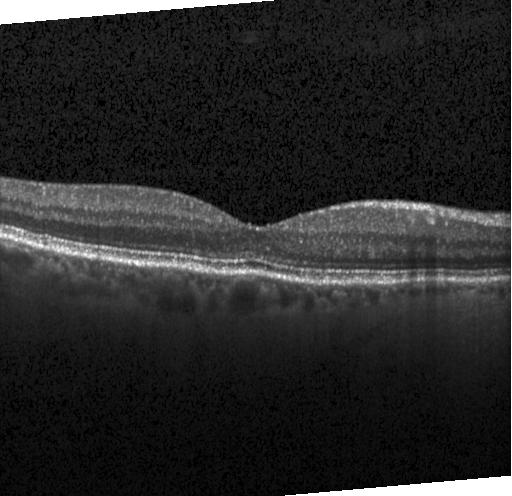

Centered on the fovea; optical coherence tomography B-scan — This B-scan demonstrates neither choroidal neovascularization, diabetic macular edema, nor drusen.